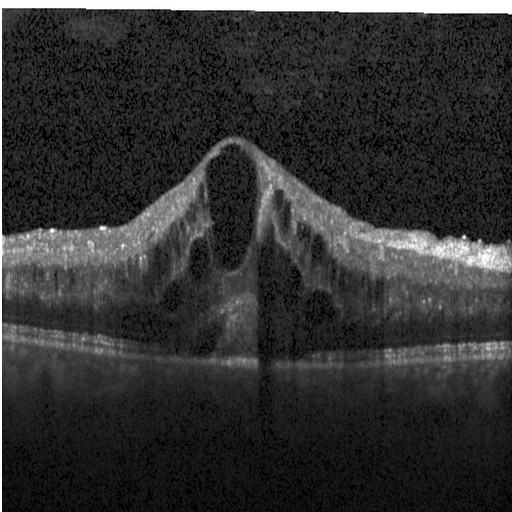 Retinal OCT B-scan. Instrument: Heidelberg Spectralis.
Diabetic macular edema (DME).